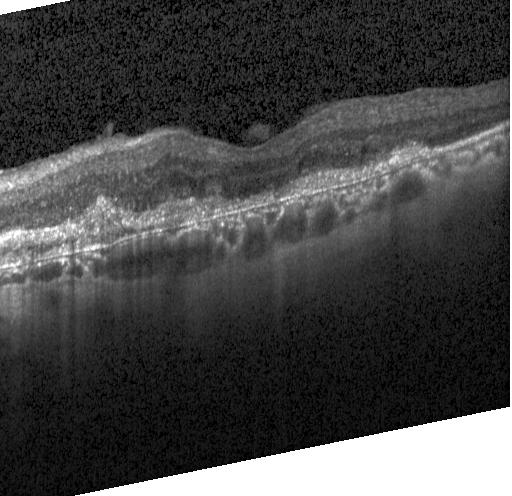
Optical coherence tomography scan.
Diagnosis: a choroidal neovascular membrane.